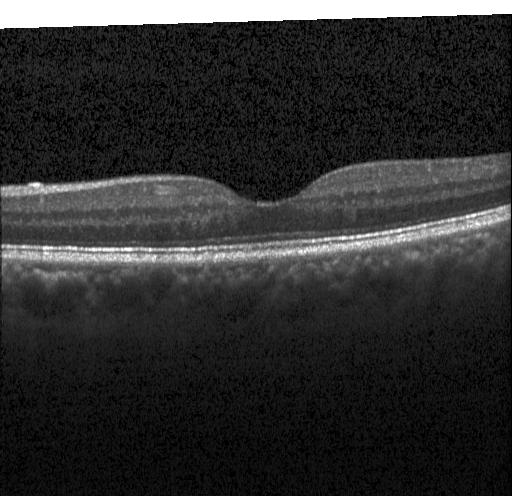
OCT B-scan, Heidelberg Spectralis — Assessment: no evidence of choroidal neovascularization, diabetic macular edema, or drusen.